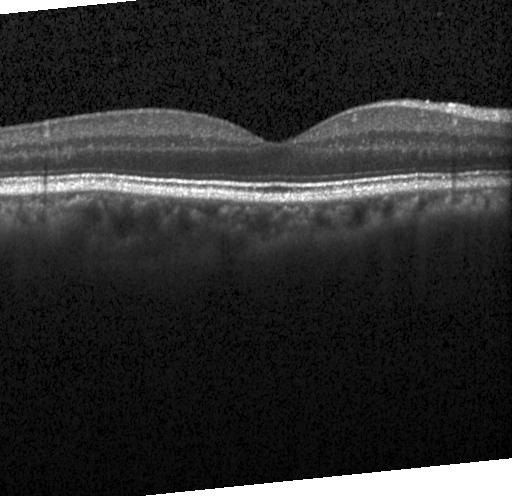
OCT scan showing neither choroidal neovascularization, diabetic macular edema, nor drusen.